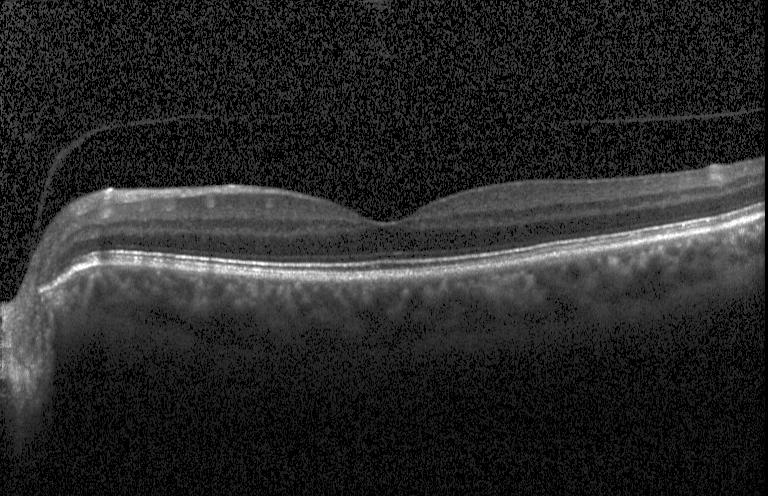 Retinal OCT B-scan. Finding: no choroidal neovascularization, no diabetic macular edema, and no drusen.